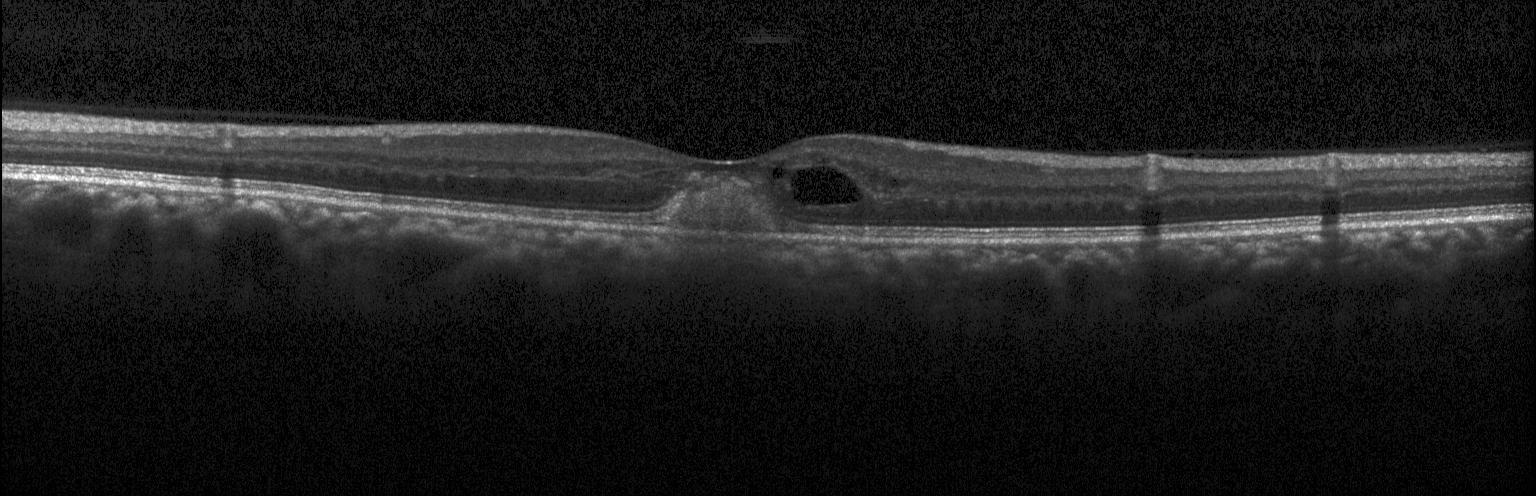 Spectral-domain OCT B-scan: CNV.